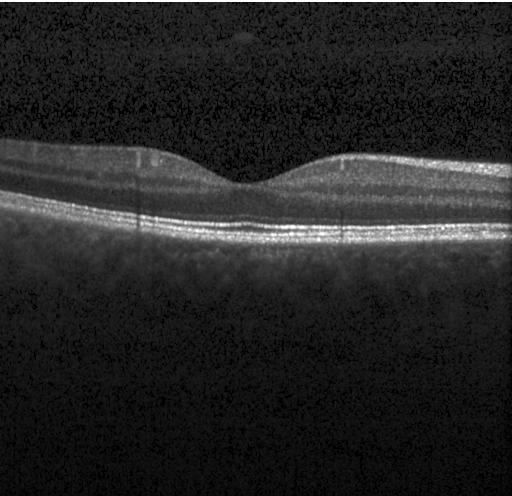 The scan shows no evidence of choroidal neovascularization, diabetic macular edema, or drusen.